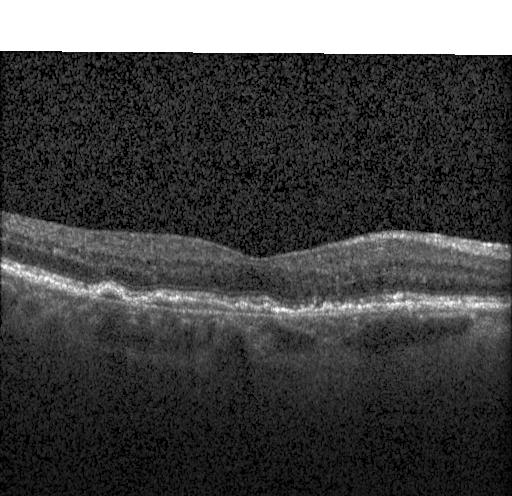
Optical coherence tomography B-scan. A choroidal neovascular membrane.